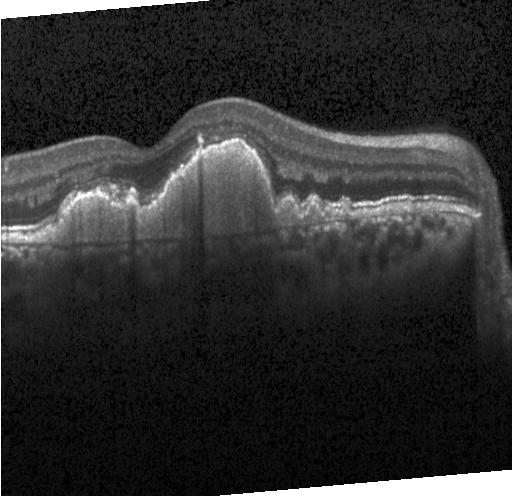
Fovea-centered, Heidelberg Spectralis, spectral-domain optical coherence tomography, optical coherence tomography B-scan. Finding: drusen.